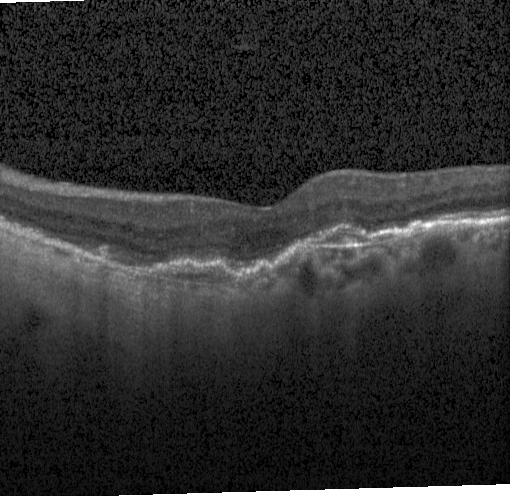
Retinal OCT cross-section. Assessment: a choroidal neovascular membrane.